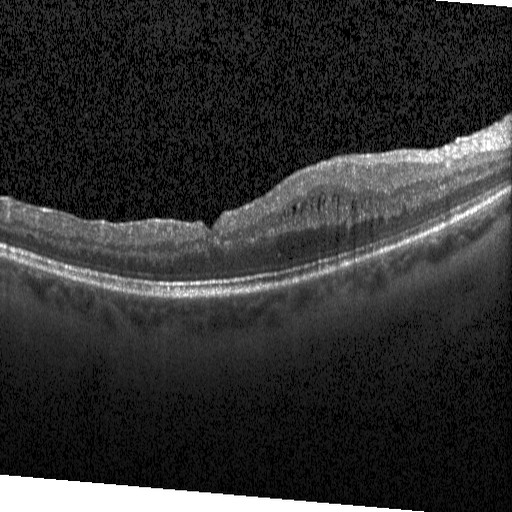 Centered on the fovea. Heidelberg Spectralis. OCT B-scan — Diagnosis: DME.